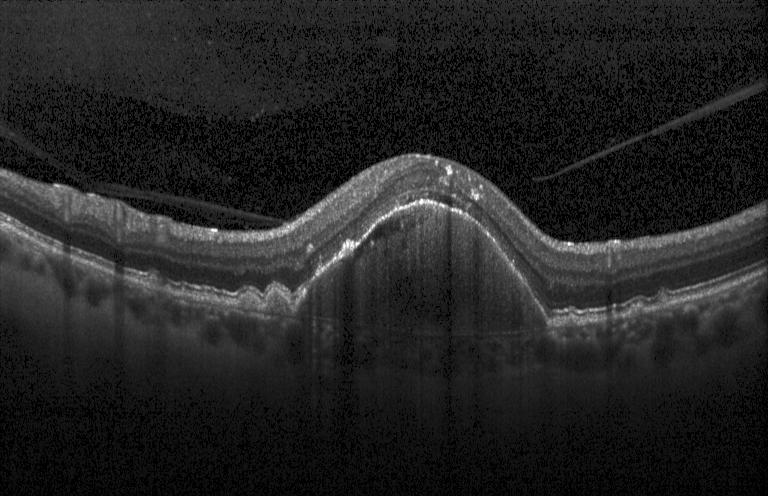

Spectral-domain OCT · macular scan · OCT line scan.
Finding: CNV.